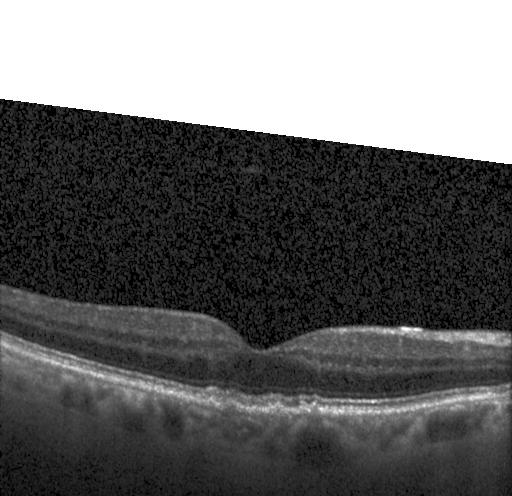 Retinal OCT B-scan · spectral-domain optical coherence tomography · Heidelberg Spectralis OCT system
The scan shows sub-RPE drusenoid deposits.